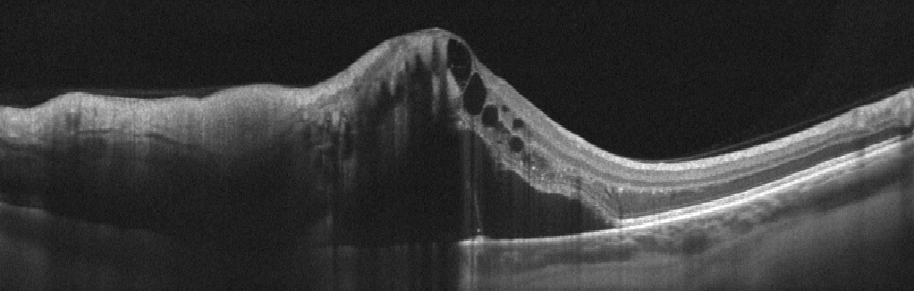
Finding: retinal vein occlusion (RVO).